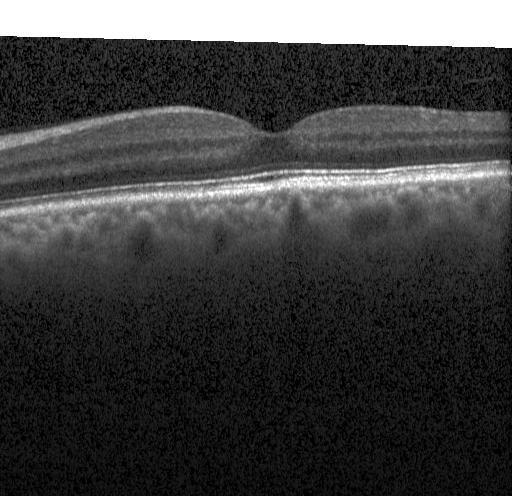
Retinal OCT B-scan. Finding: neither choroidal neovascularization, diabetic macular edema, nor drusen.